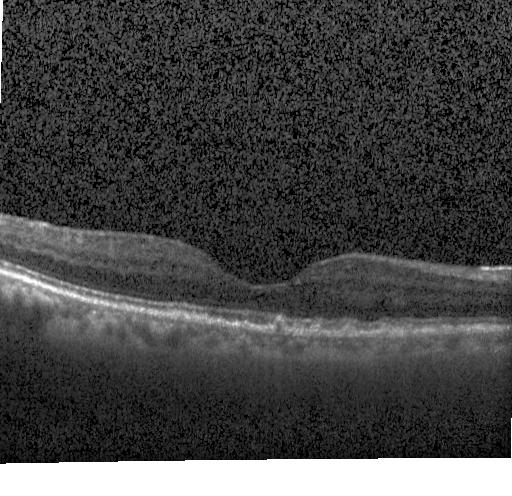
Assessment: multiple drusen.